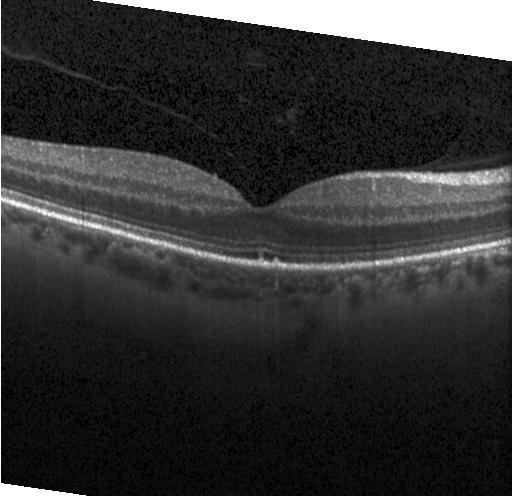
Diagnosis: multiple drusen.